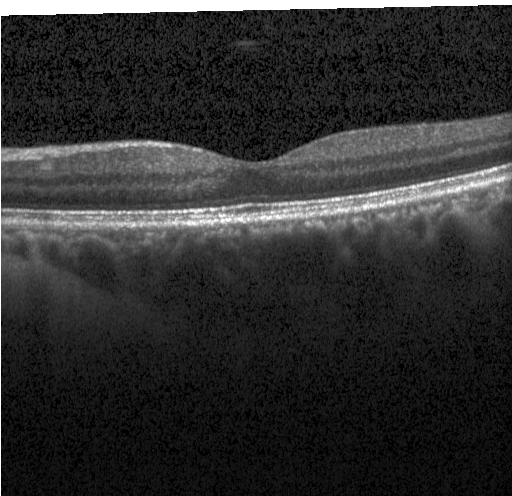 OCT B-scan showing no CNV, no DME, and no drusen.